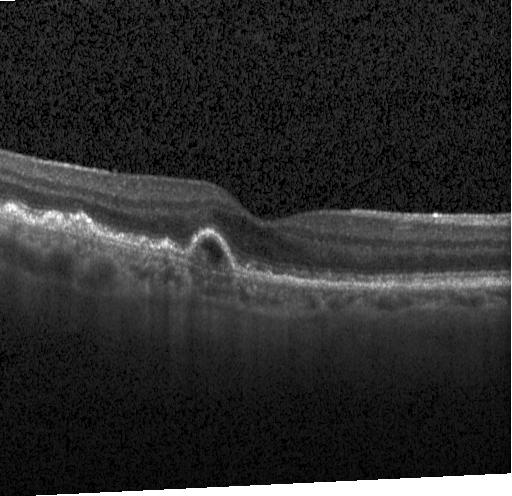

Retinal OCT B-scan.
Finding: multiple drusen.